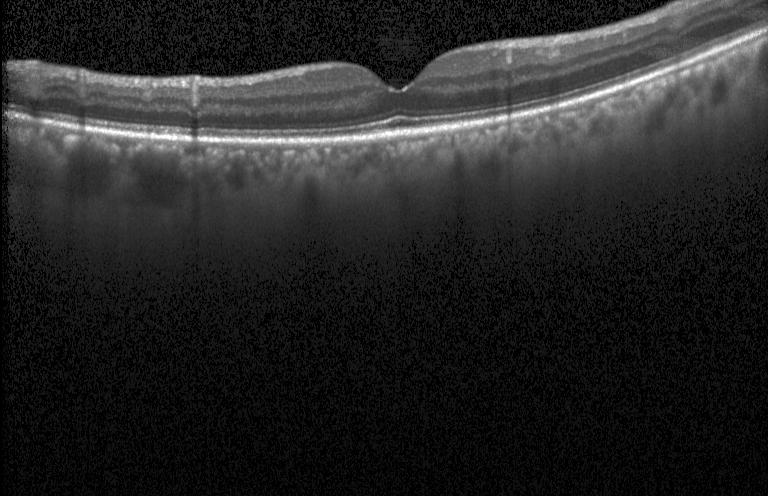

OCT line scan — Finding: no CNV, no DME, and no drusen.